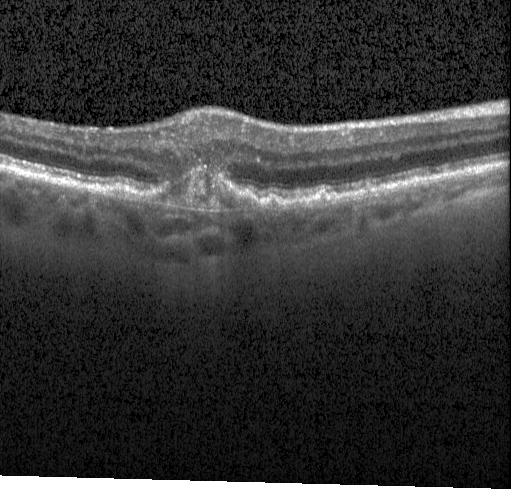 Spectral-domain optical coherence tomography, optical coherence tomography B-scan, acquired on a Heidelberg Spectralis.
Dx: a choroidal neovascular membrane.